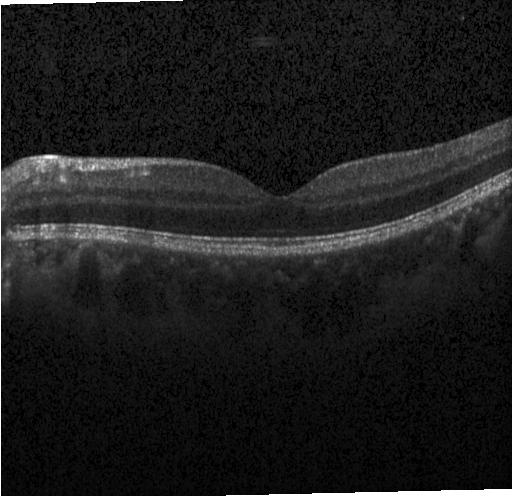
Macular OCT demonstrating no evidence of choroidal neovascularization, diabetic macular edema, or drusen.